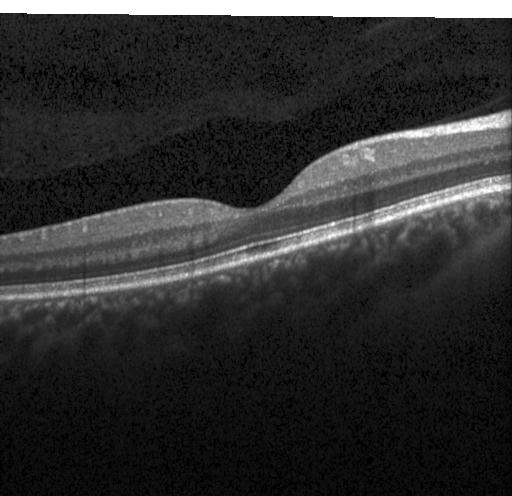

The scan shows no choroidal neovascularization, diabetic macular edema, or drusen.